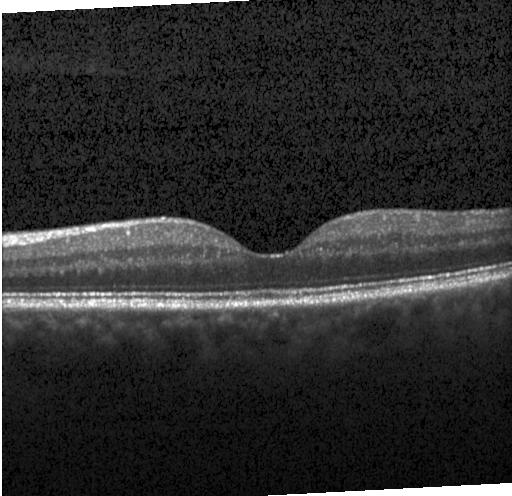

Spectral-domain OCT. Retinal OCT cross-section.
Dx: no choroidal neovascularization, diabetic macular edema, or drusen.